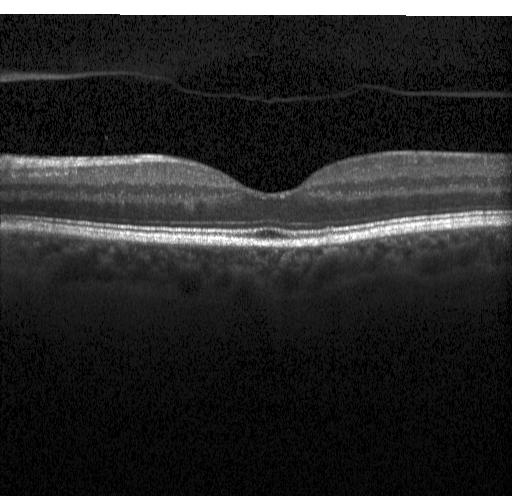
Horizontal scan through the fovea · SD-OCT · instrument: Heidelberg Spectralis · OCT line scan. The scan shows no choroidal neovascularization, diabetic macular edema, or drusen.